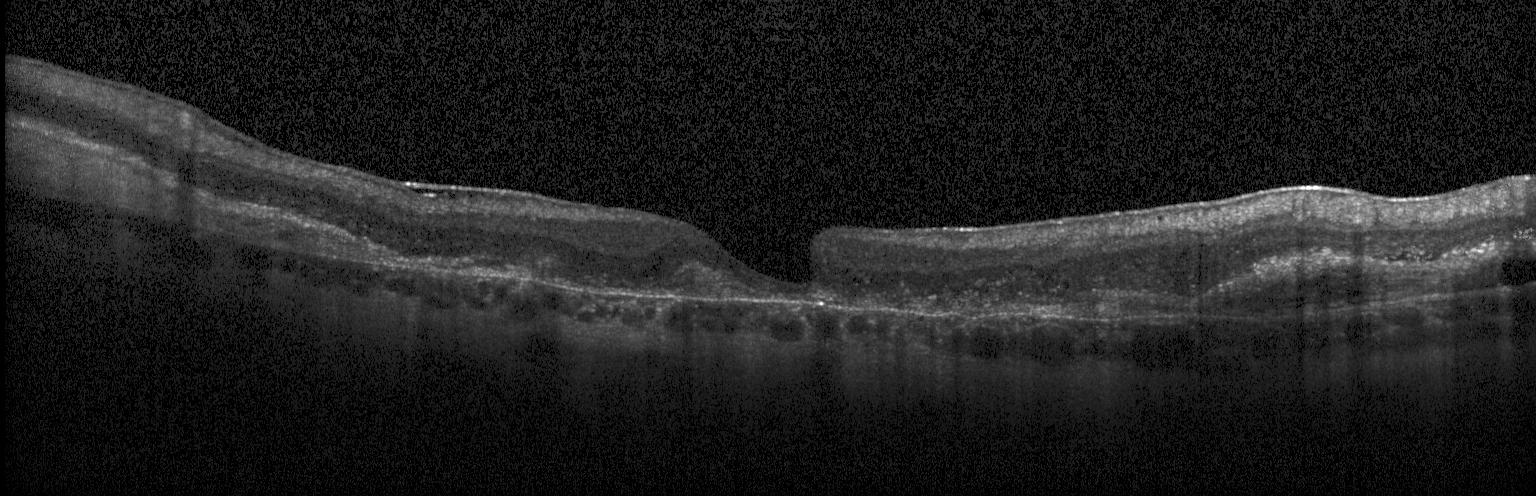
Optical coherence tomography scan
Diagnosis: choroidal neovascularization (CNV).